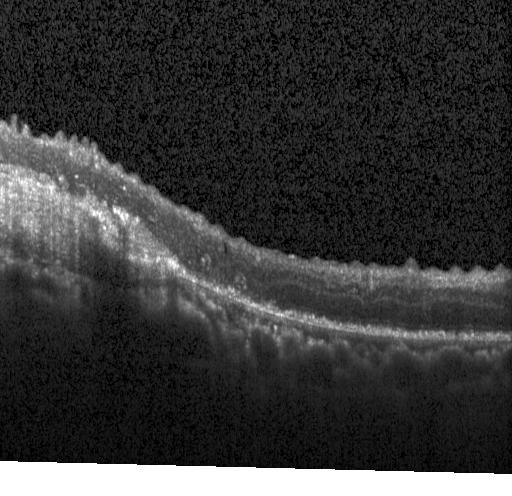
OCT line scan, centered on the fovea, SD-OCT — Diagnosis: a choroidal neovascular membrane.